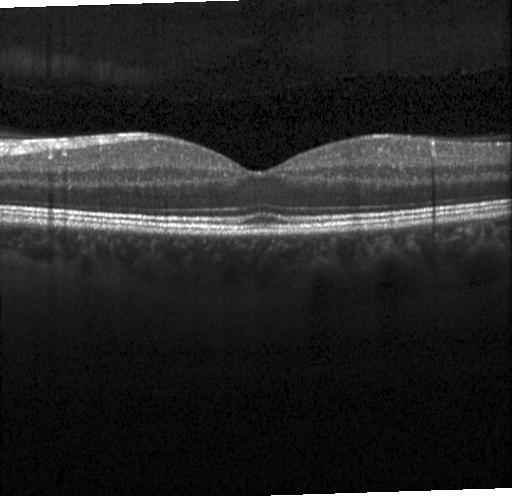 Retinal OCT B-scan.
Dx: no evidence of CNV, DME, or drusen.